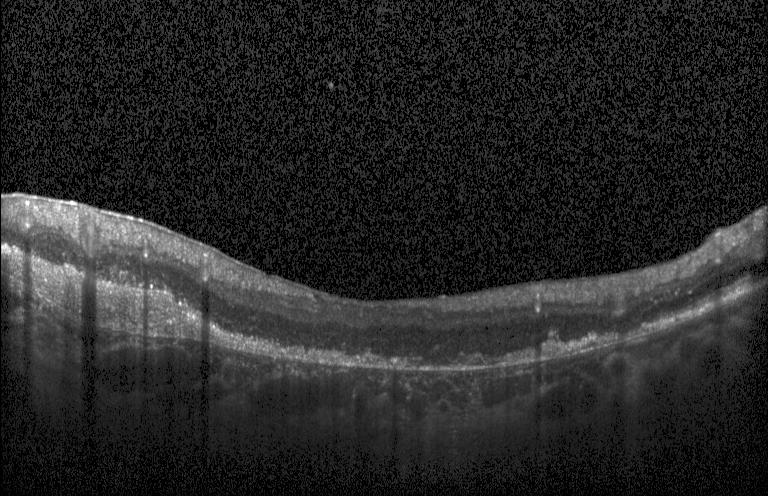
Impression: CNV.